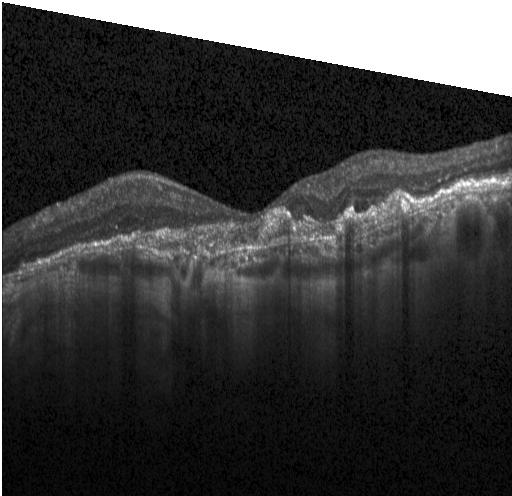

Horizontal scan through the fovea. Retinal OCT cross-section. Acquired on a Heidelberg Spectralis
Impression: choroidal neovascularization.